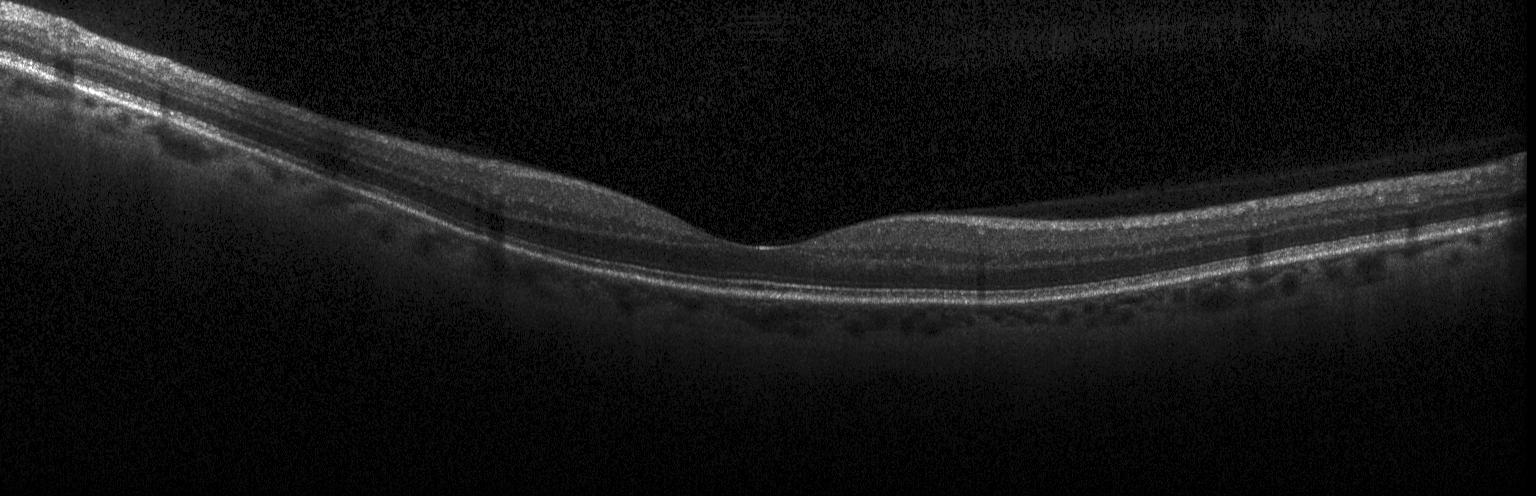 Retinal OCT B-scan · Heidelberg Spectralis · spectral-domain optical coherence tomography · horizontal scan through the fovea. Finding: no choroidal neovascularization, diabetic macular edema, or drusen.